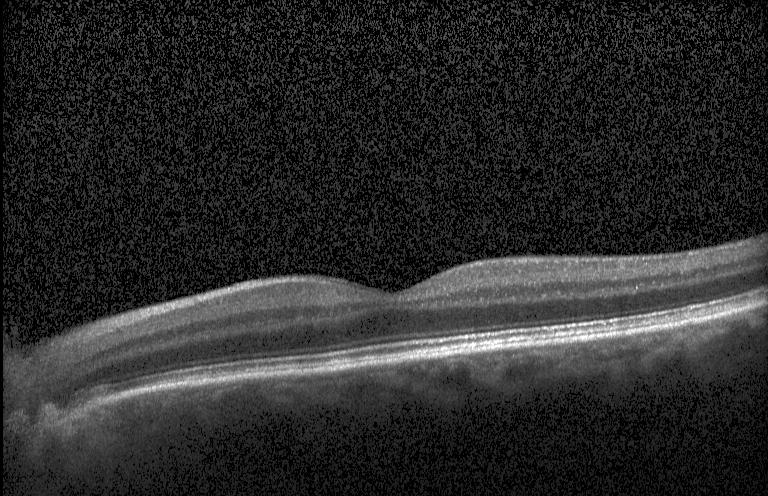

Macular OCT demonstrating no CNV, no DME, and no drusen.